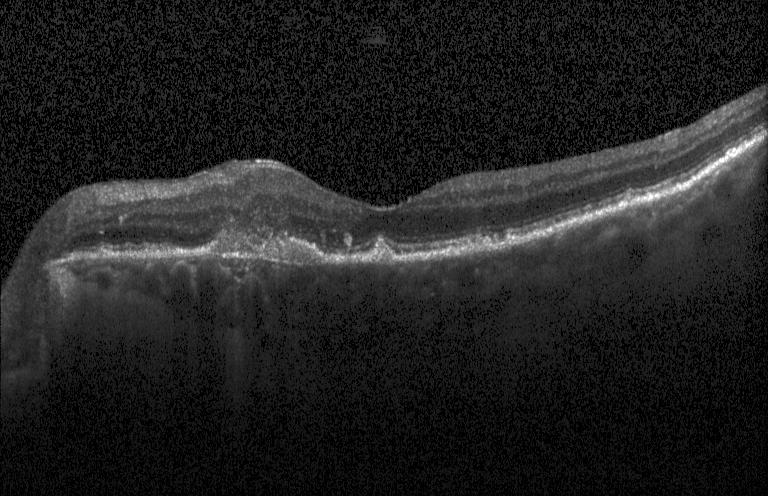
Heidelberg Spectralis OCT system, spectral-domain OCT, through the macula, OCT B-scan.
Finding: CNV.